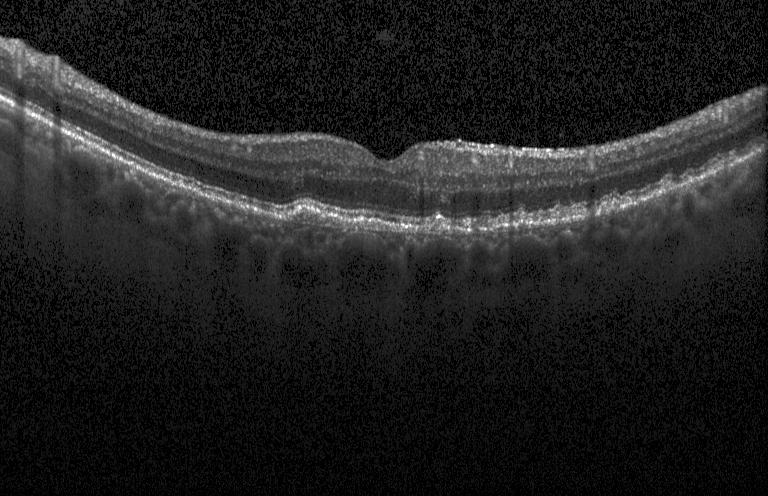
OCT B-scan. Spectral-domain OCT. Centered on the fovea. Acquired on a Heidelberg Spectralis
Impression: a choroidal neovascular membrane.